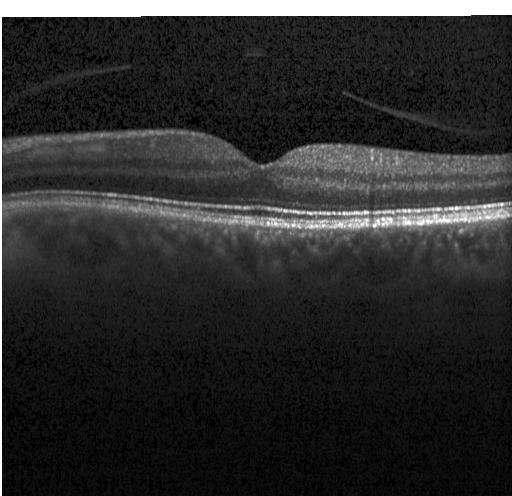
Impression: no choroidal neovascularization, diabetic macular edema, or drusen.